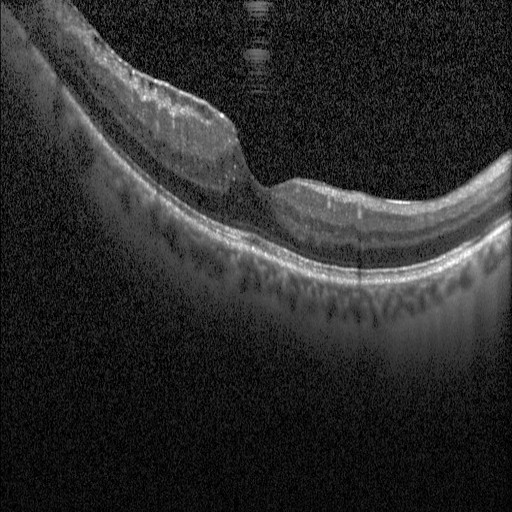 Optical coherence tomography B-scan.
Assessment: DME.